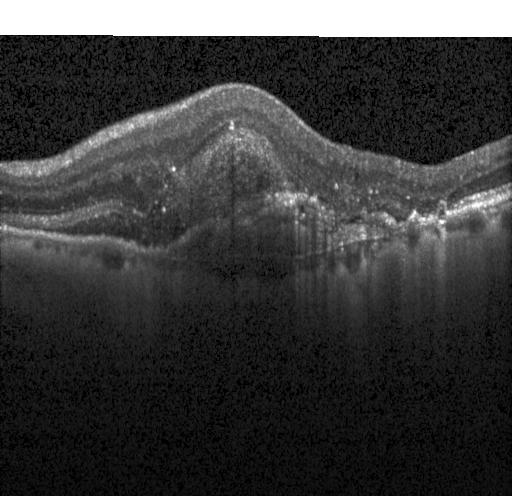 This B-scan demonstrates CNV.